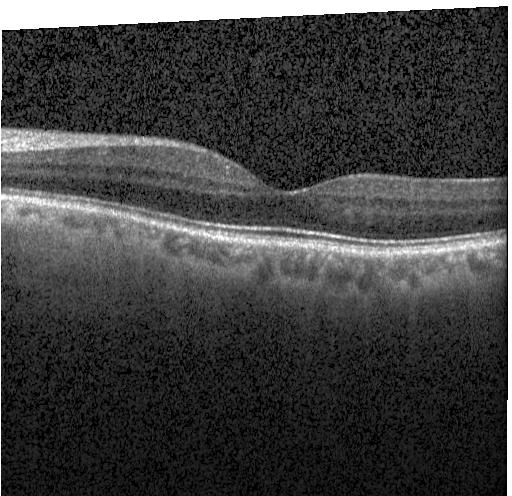 Acquired on a Heidelberg Spectralis. OCT B-scan. SD-OCT. Fovea-centered
No evidence of choroidal neovascularization, diabetic macular edema, or drusen.